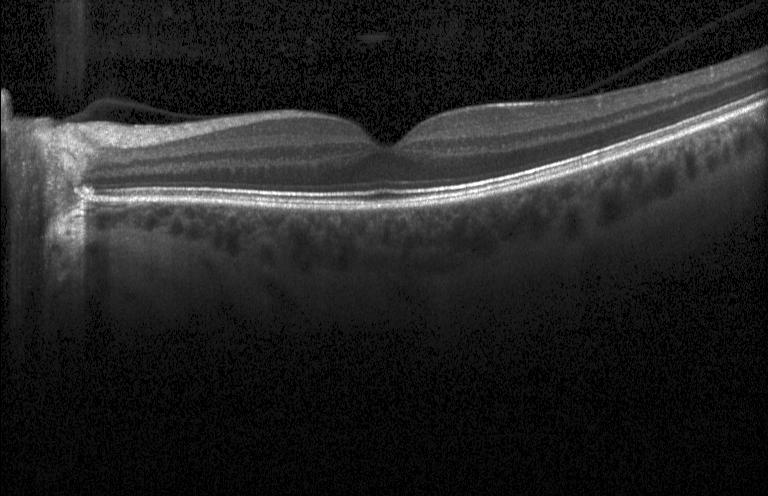

Heidelberg Spectralis, horizontal scan through the fovea, retinal OCT cross-section — This B-scan demonstrates no evidence of choroidal neovascularization, diabetic macular edema, or drusen.